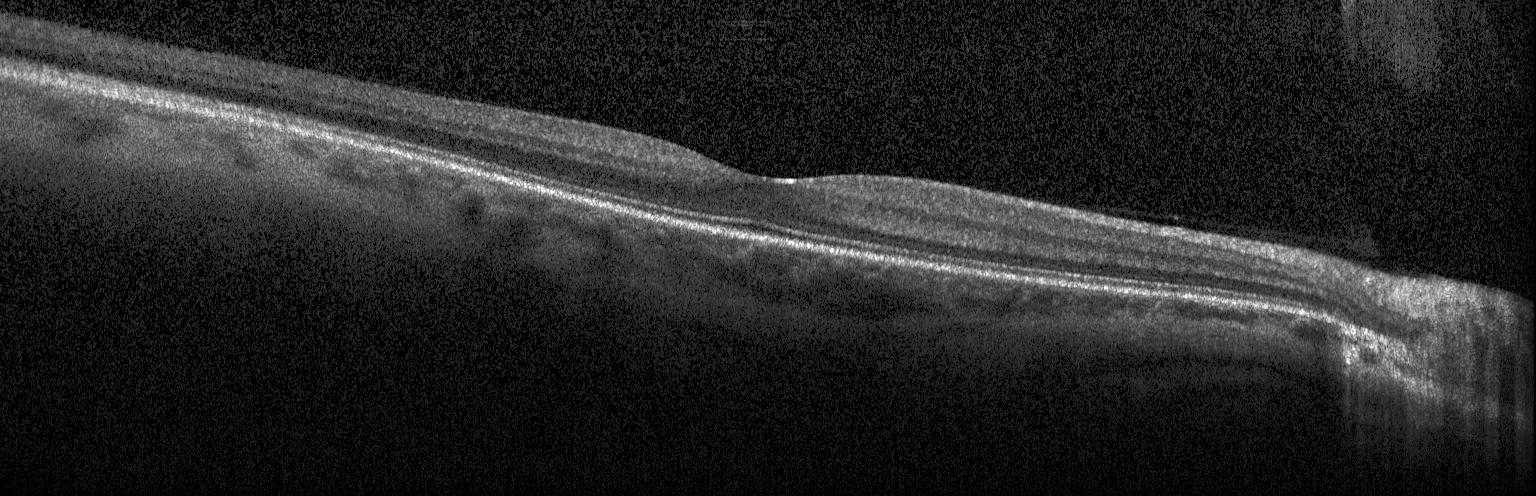
Retinal OCT B-scan. Impression: no evidence of choroidal neovascularization, diabetic macular edema, or drusen.